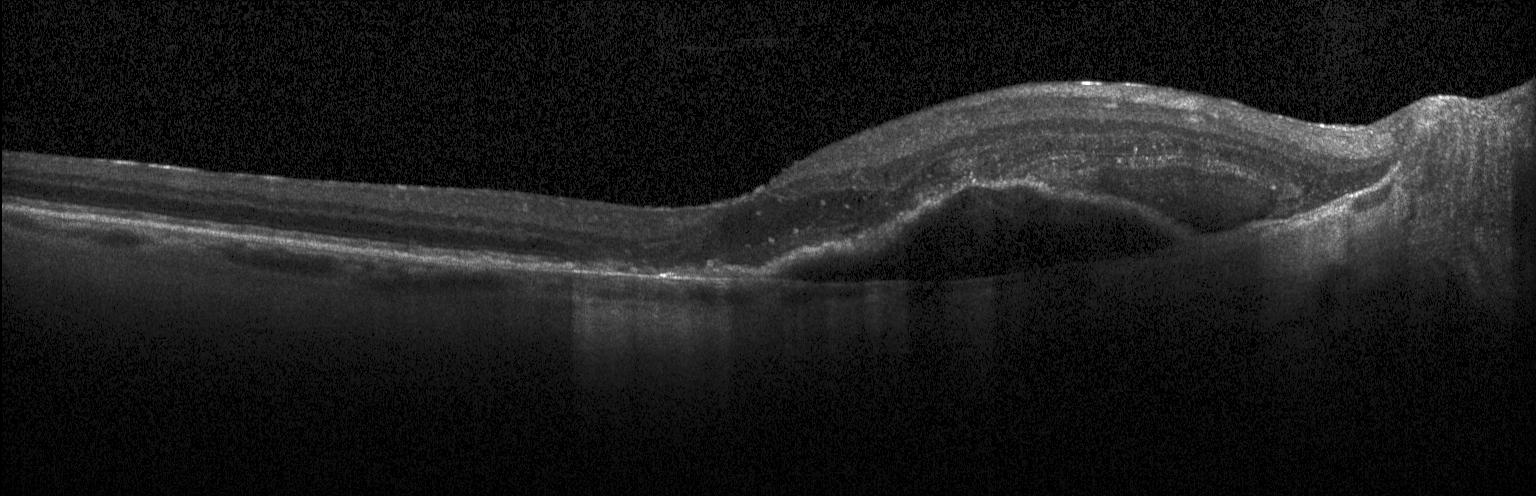
Optical coherence tomography scan.
A choroidal neovascular membrane.